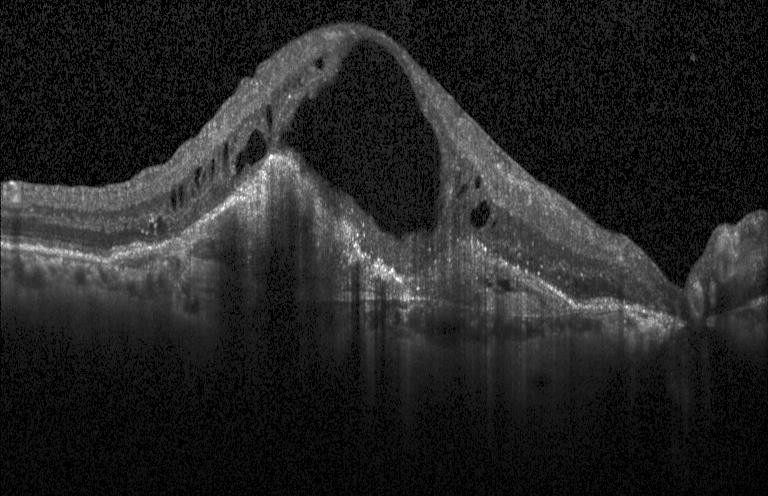 Through the macula. Spectral-domain optical coherence tomography. Retinal OCT cross-section. Diagnosis: CNV.